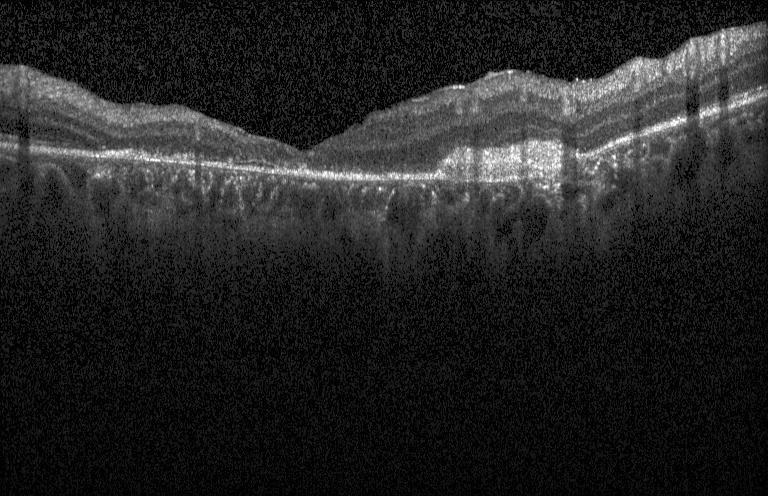

Fovea-centered; Heidelberg Spectralis; spectral-domain optical coherence tomography; retinal OCT B-scan.
Diagnosis: CNV.